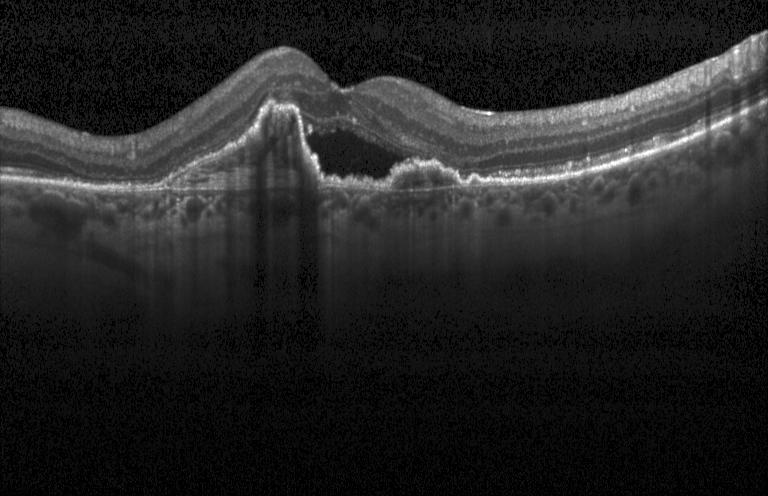
Finding: a choroidal neovascular membrane.